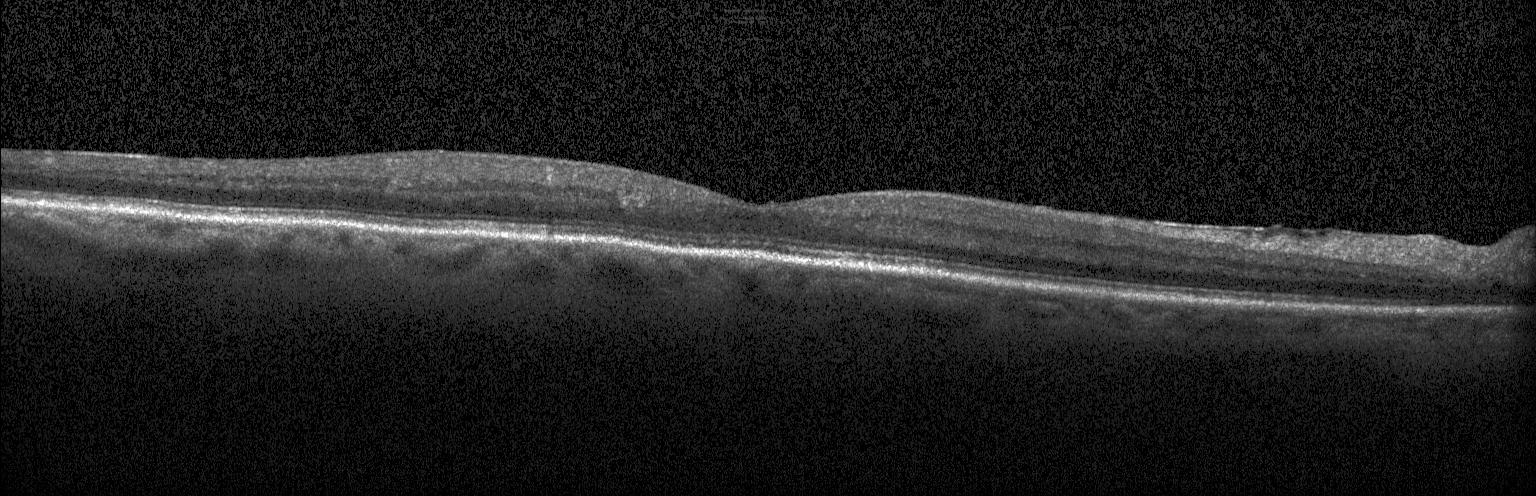 OCT line scan. Spectral-domain optical coherence tomography — This B-scan demonstrates no evidence of choroidal neovascularization, diabetic macular edema, or drusen.